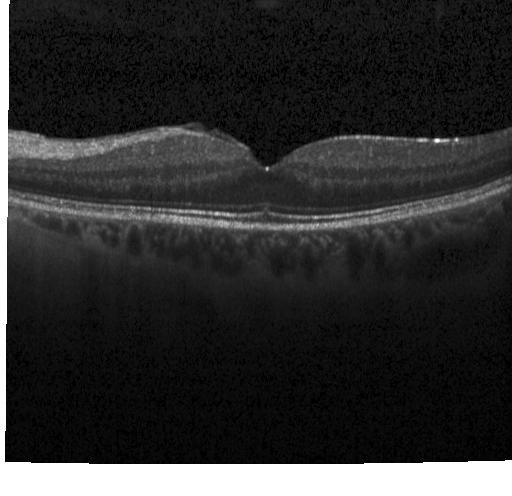

Spectral-domain optical coherence tomography, retinal OCT B-scan, acquired on a Heidelberg Spectralis. Assessment: no choroidal neovascularization, diabetic macular edema, or drusen.